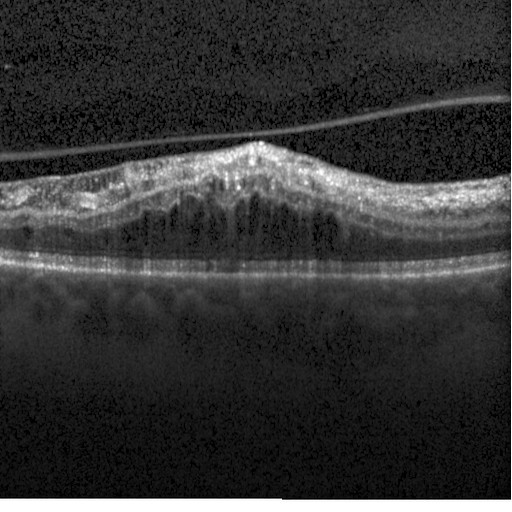

Optical coherence tomography scan; centered on the fovea; spectral-domain OCT; Heidelberg Spectralis. Finding: DME.